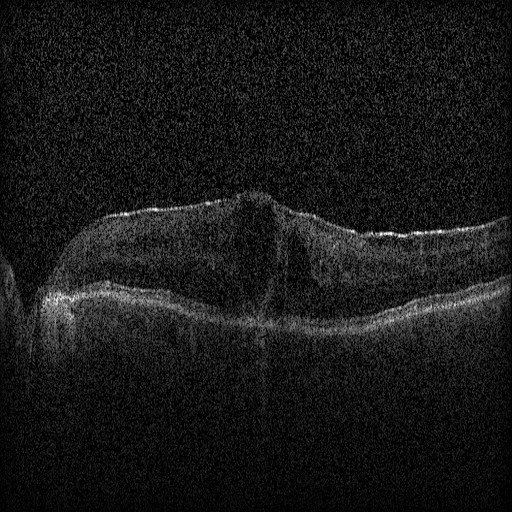

The scan shows DME.